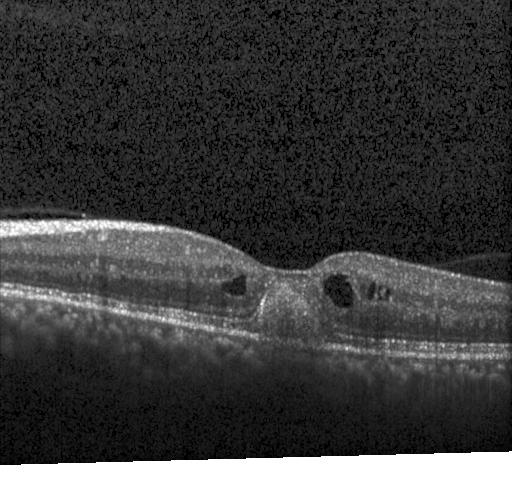

Spectral-domain optical coherence tomography · OCT B-scan.
Macular OCT: a choroidal neovascular membrane.